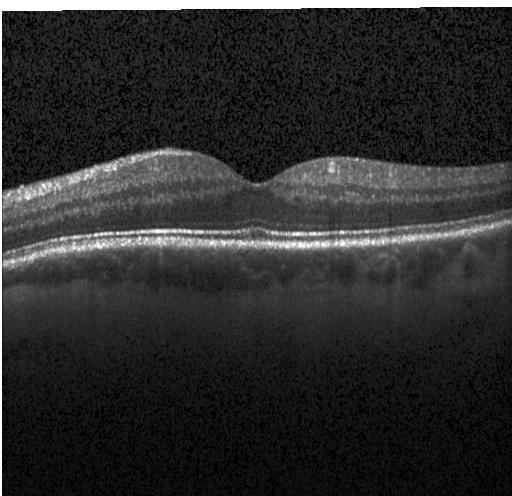 OCT line scan; instrument: Heidelberg Spectralis; spectral-domain optical coherence tomography — No evidence of choroidal neovascularization, diabetic macular edema, or drusen.